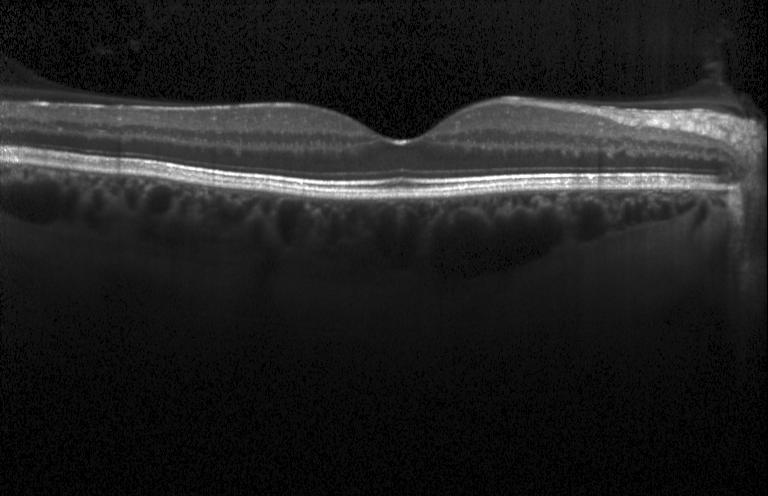 Acquired on a Heidelberg Spectralis. Spectral-domain optical coherence tomography. Through the macula. Optical coherence tomography scan.
No choroidal neovascularization, no diabetic macular edema, and no drusen.